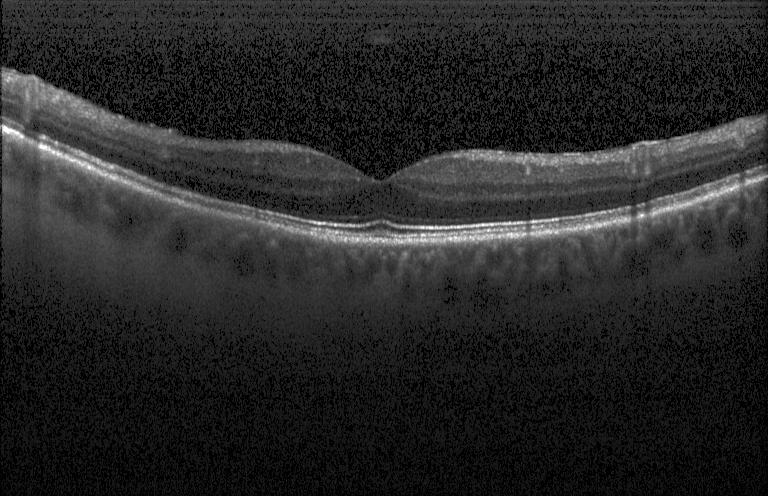 Heidelberg Spectralis OCT system. OCT B-scan. Horizontal scan through the fovea — Diagnosis: no choroidal neovascularization, diabetic macular edema, or drusen.